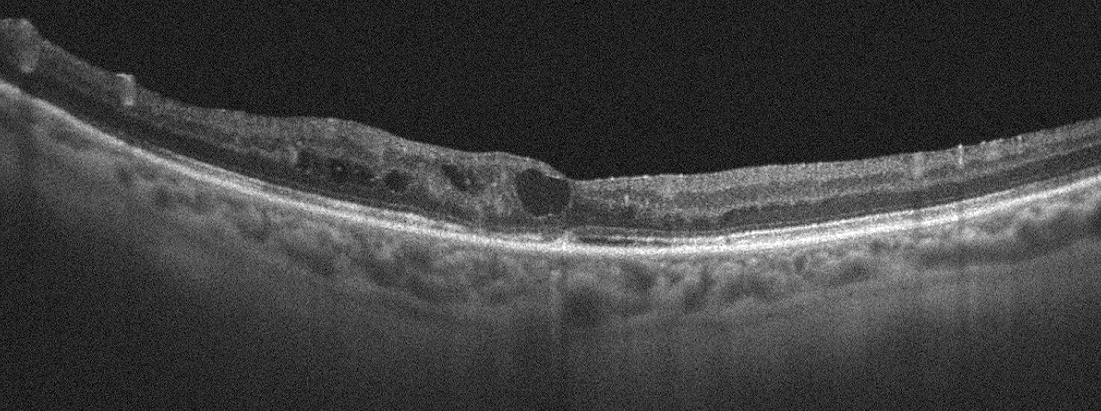 Macular OCT demonstrating diabetic macular edema.